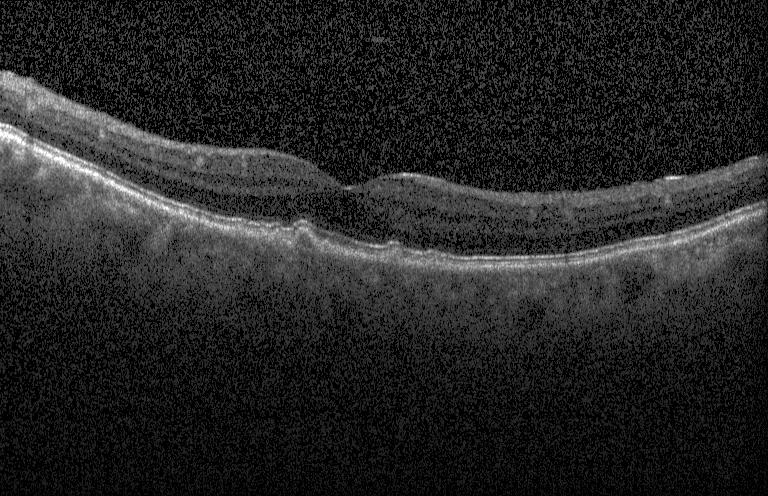

Spectral-domain optical coherence tomography · through the macula · instrument: Heidelberg Spectralis · OCT line scan. Impression: sub-RPE drusenoid deposits.